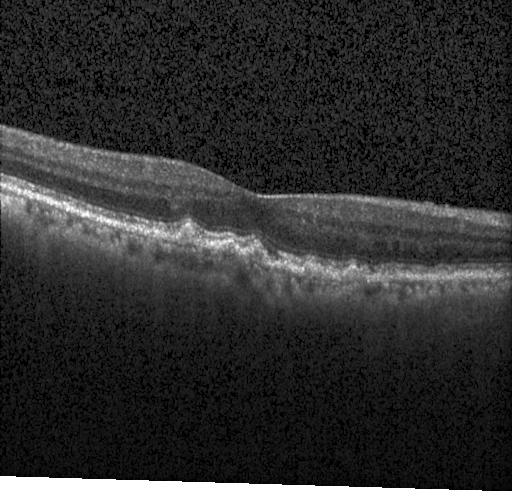

Impression: drusen.